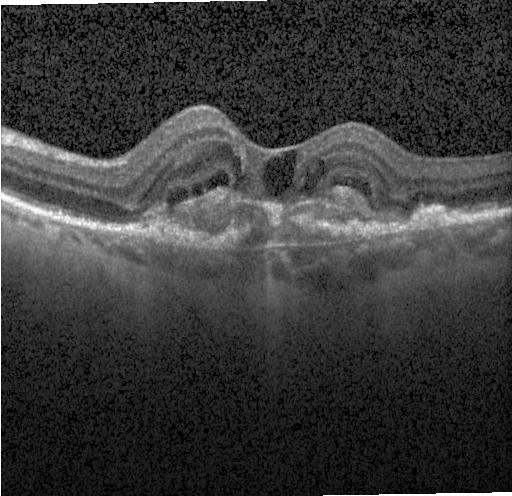

Macular OCT: choroidal neovascularization.